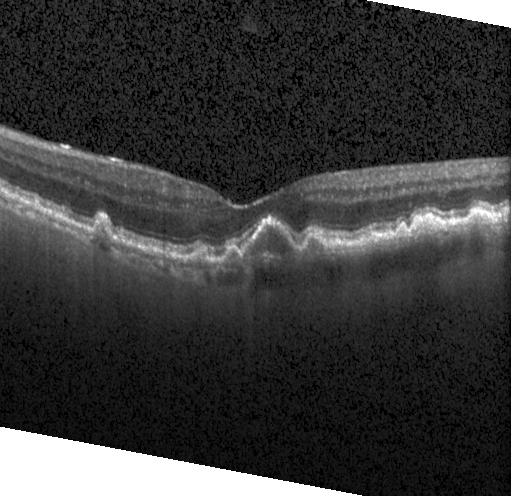
Optical coherence tomography B-scan. SD-OCT. Acquired on a Heidelberg Spectralis. Impression: sub-RPE drusenoid deposits.